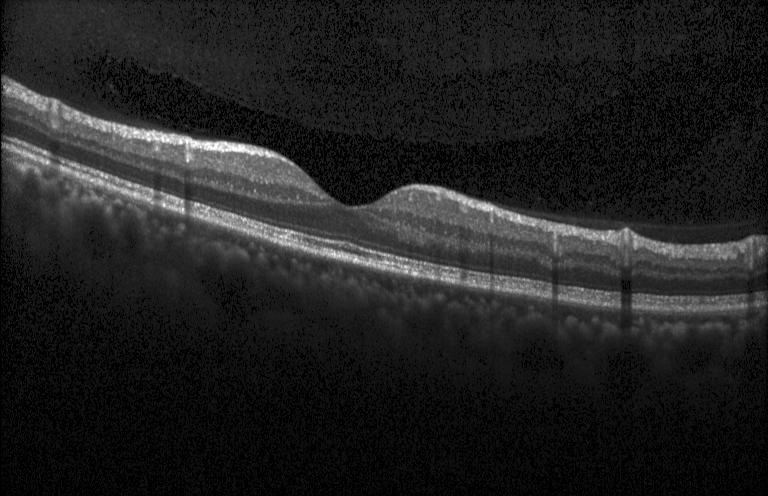
Impression: no choroidal neovascularization, no diabetic macular edema, and no drusen.